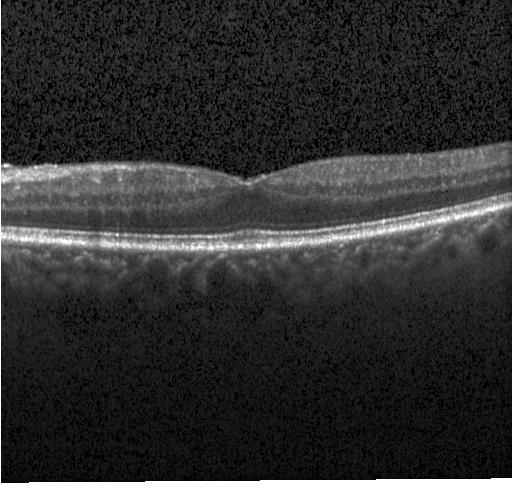
Diagnosis: no evidence of CNV, DME, or drusen.